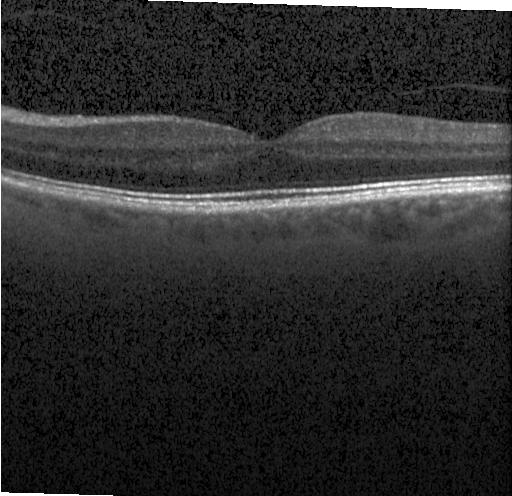

OCT line scan; SD-OCT; acquired on a Heidelberg Spectralis; fovea-centered.
Finding: no evidence of CNV, DME, or drusen.